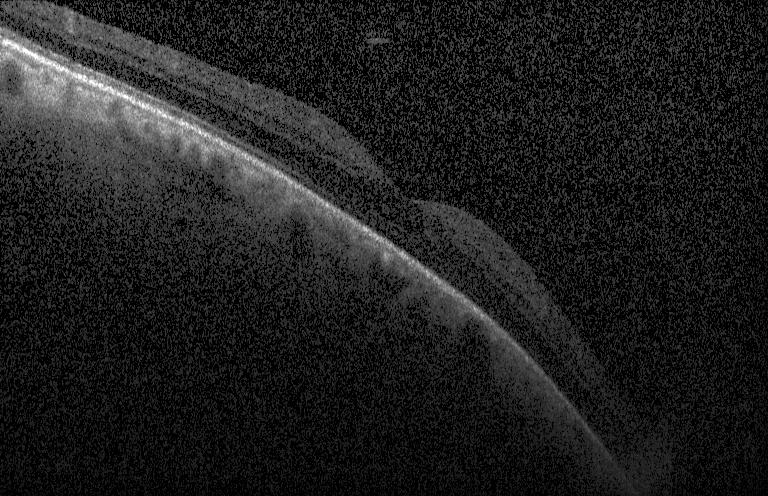

Retinal OCT cross-section, SD-OCT, through the macula, acquired on a Heidelberg Spectralis
Assessment: no evidence of CNV, DME, or drusen.